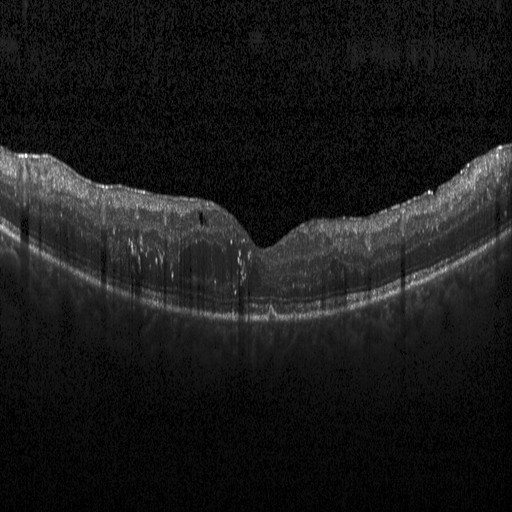 Diagnosis: diabetic macular edema.